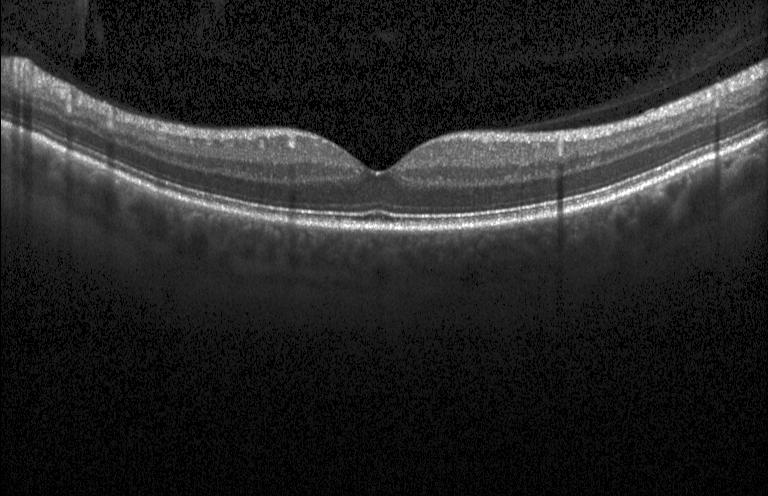
Spectral-domain OCT · retinal OCT cross-section — Macular OCT: neither choroidal neovascularization, diabetic macular edema, nor drusen.